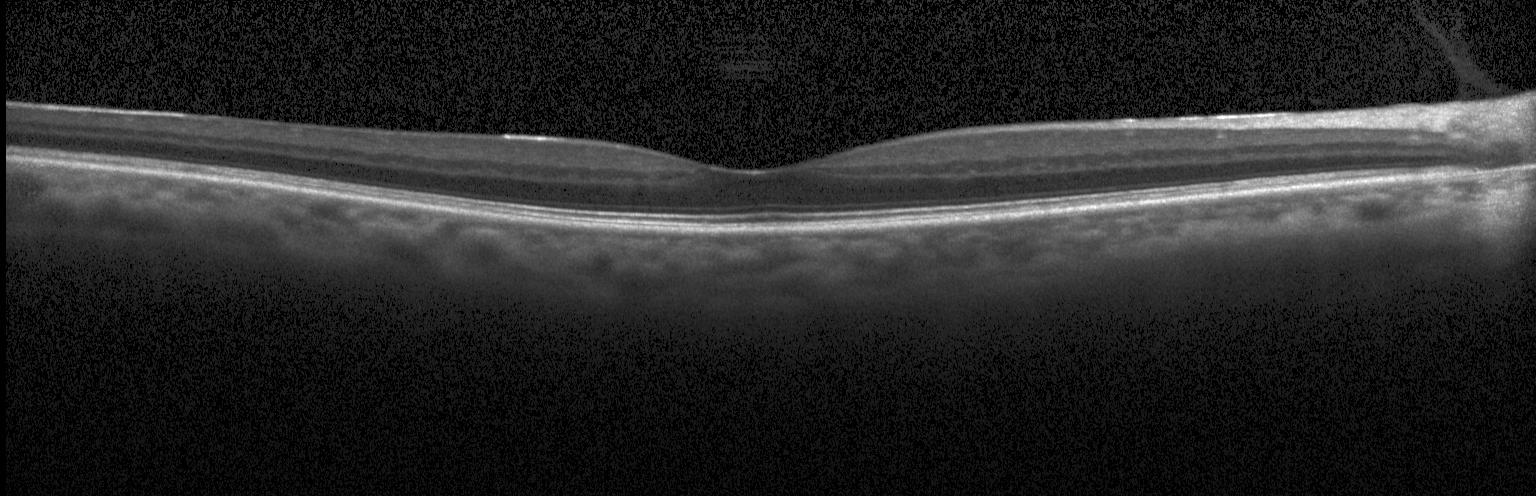

Instrument: Heidelberg Spectralis · OCT line scan · through the macula. Impression: neither choroidal neovascularization, diabetic macular edema, nor drusen.